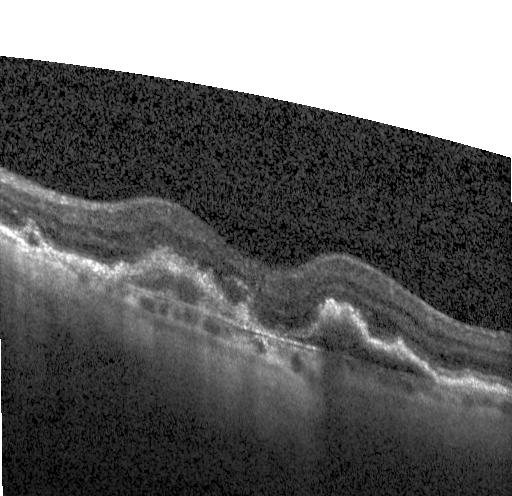
Optical coherence tomography B-scan. Choroidal neovascularization (CNV).